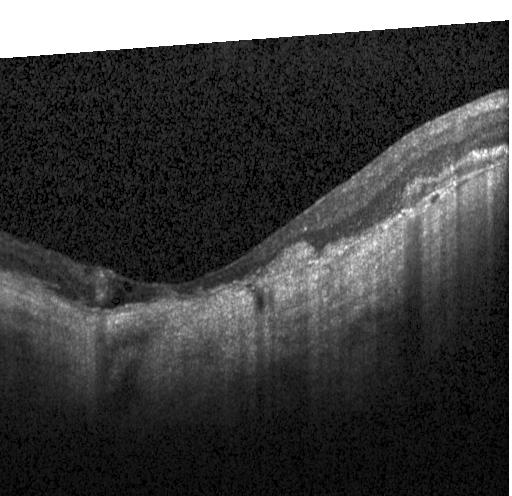

OCT scan showing a choroidal neovascular membrane.